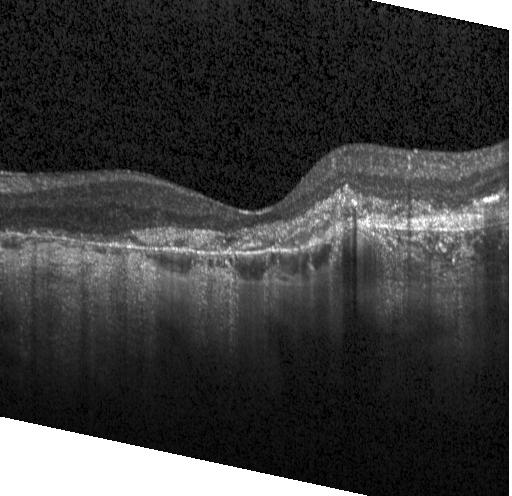 OCT scan showing choroidal neovascularization.